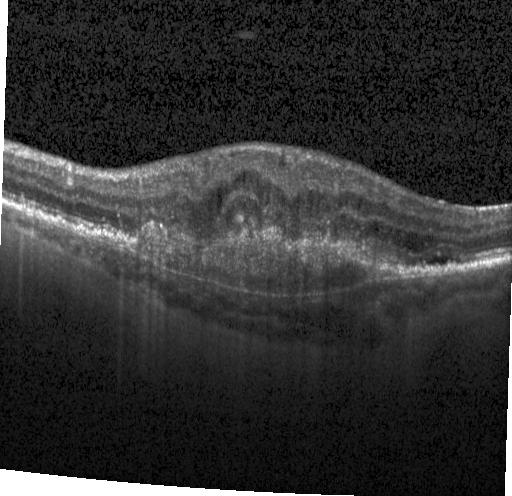

SD-OCT, retinal OCT B-scan, Heidelberg Spectralis — The scan shows choroidal neovascularization.